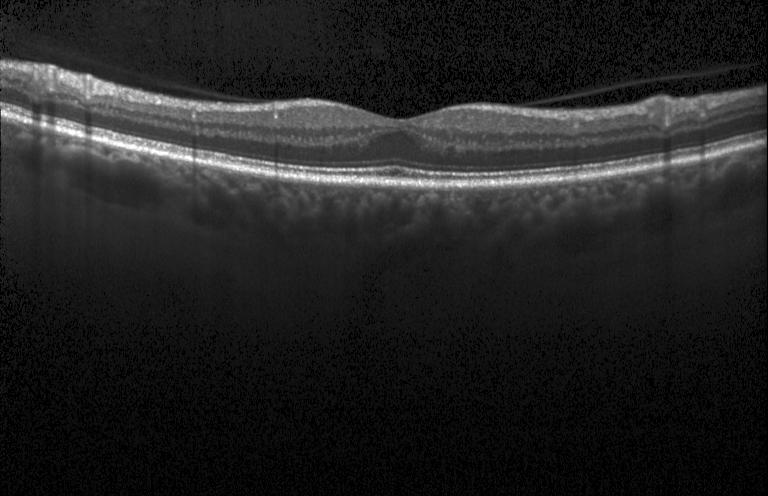
Retinal OCT B-scan
OCT finding: no choroidal neovascularization, diabetic macular edema, or drusen.